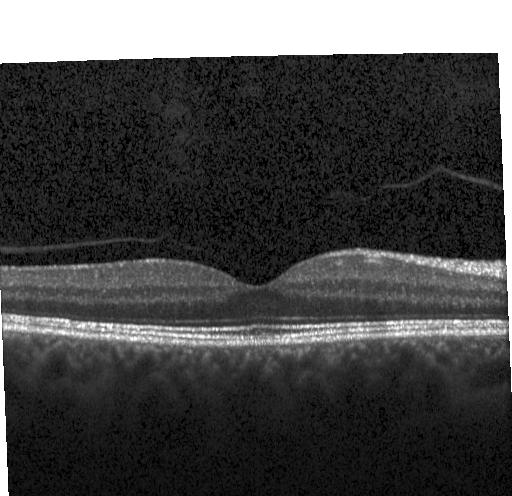

OCT finding: no evidence of choroidal neovascularization, diabetic macular edema, or drusen.